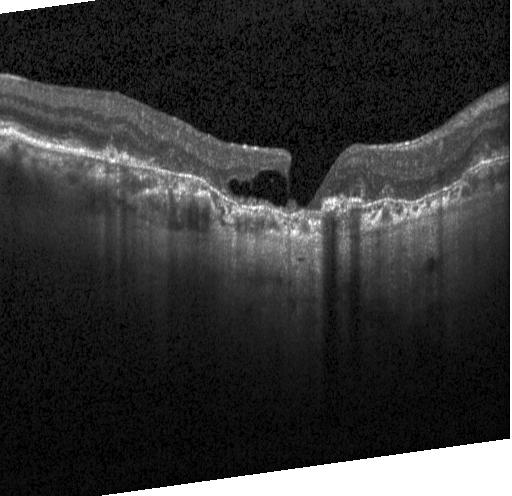
Retinal OCT B-scan, through the macula. Impression: CNV.